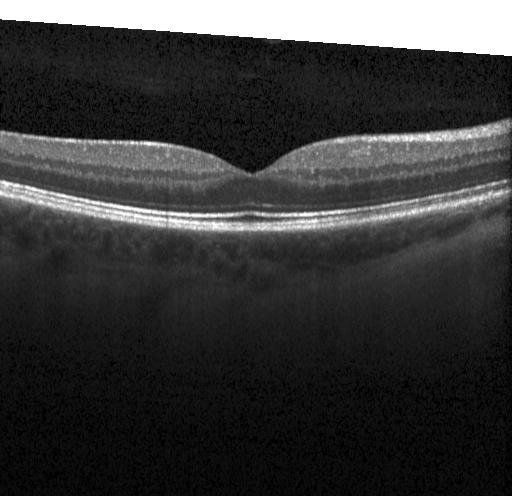 Optical coherence tomography scan. Heidelberg Spectralis. Through the macula. Impression: neither choroidal neovascularization, diabetic macular edema, nor drusen.